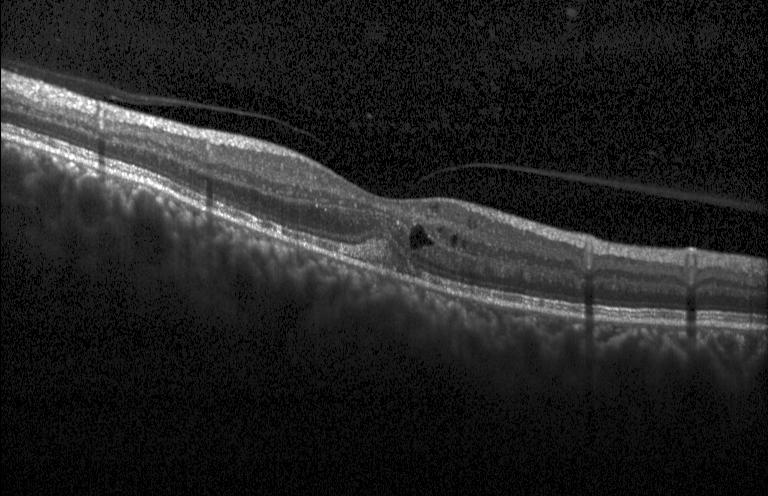 OCT B-scan.
A choroidal neovascular membrane.